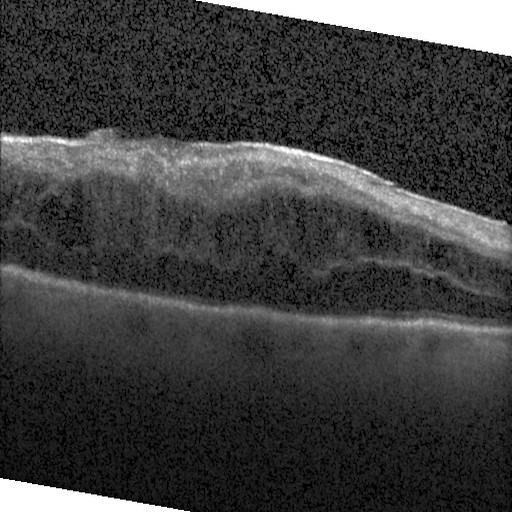

OCT line scan; macular scan; Heidelberg Spectralis; SD-OCT.
OCT finding: diabetic macular edema (DME).